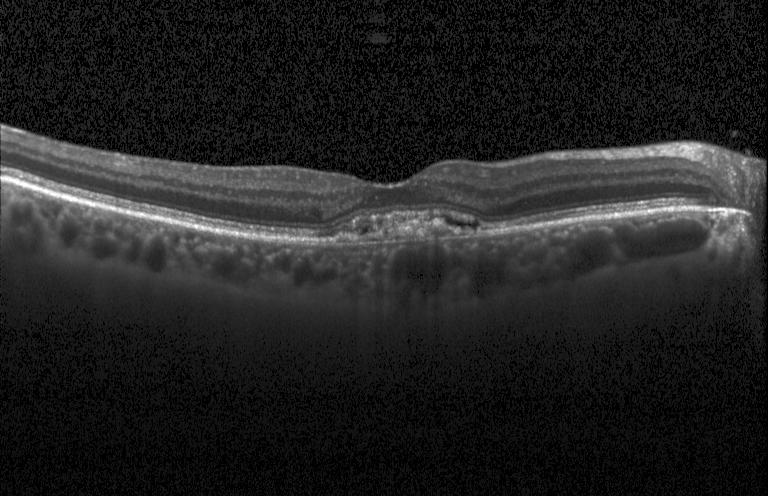
Fovea-centered; optical coherence tomography B-scan; Heidelberg Spectralis OCT system; spectral-domain optical coherence tomography — Diagnosis: a choroidal neovascular membrane.